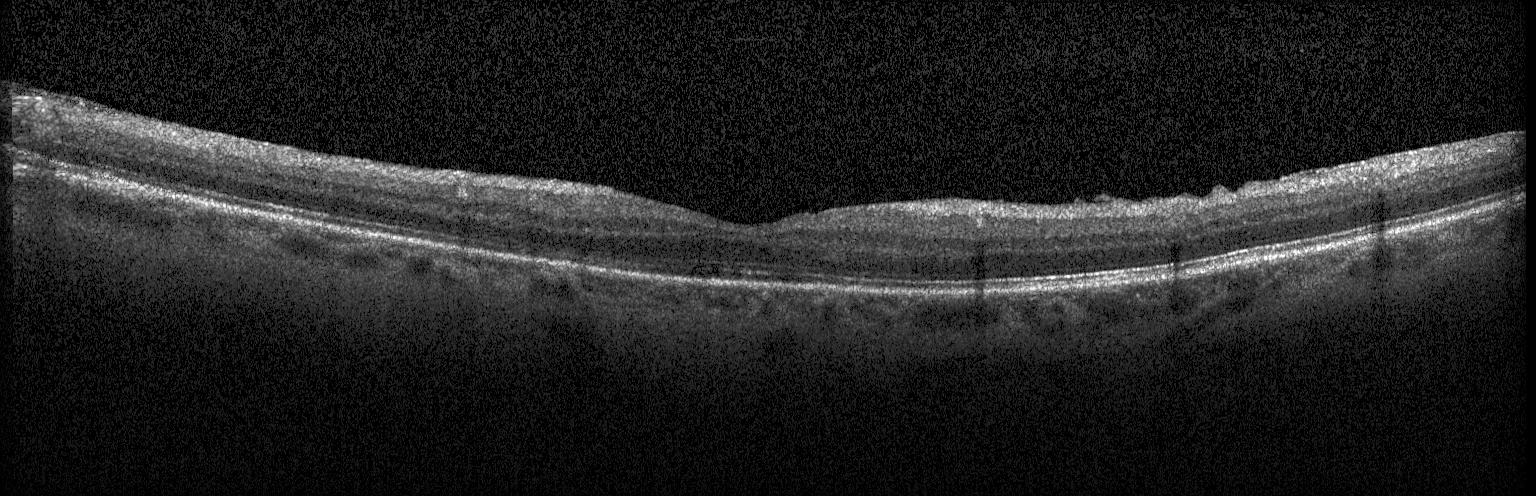
Spectral-domain OCT. Optical coherence tomography B-scan
Assessment: no choroidal neovascularization, no diabetic macular edema, and no drusen.